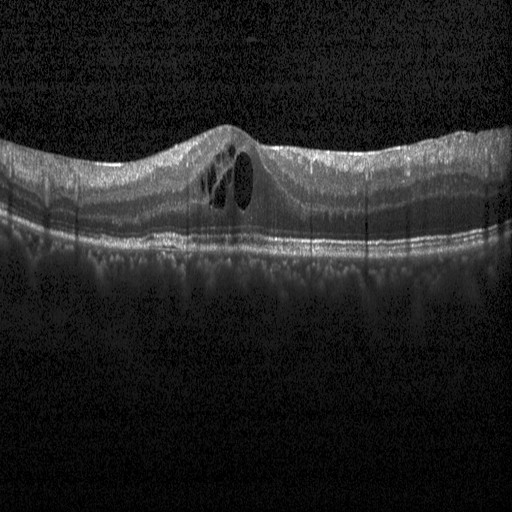

OCT finding: DME.